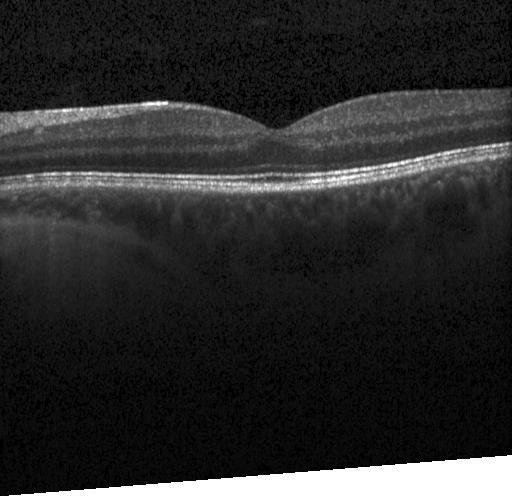 Diagnosis: no evidence of CNV, DME, or drusen.